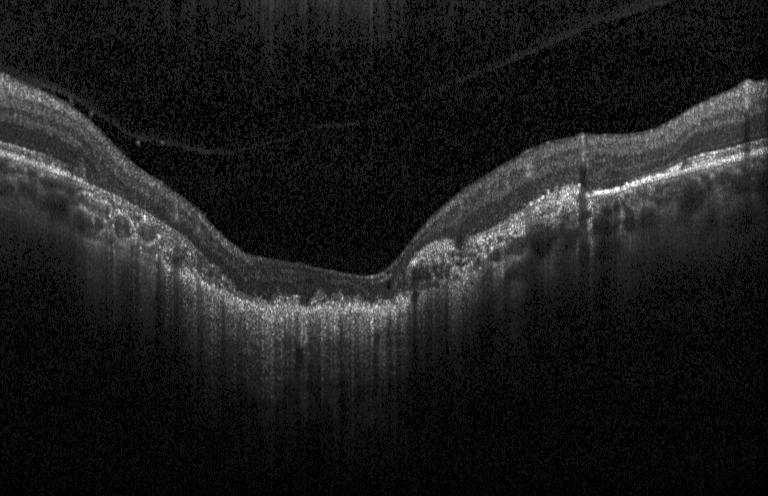 Through the macula. Retinal OCT cross-section
Choroidal neovascularization.